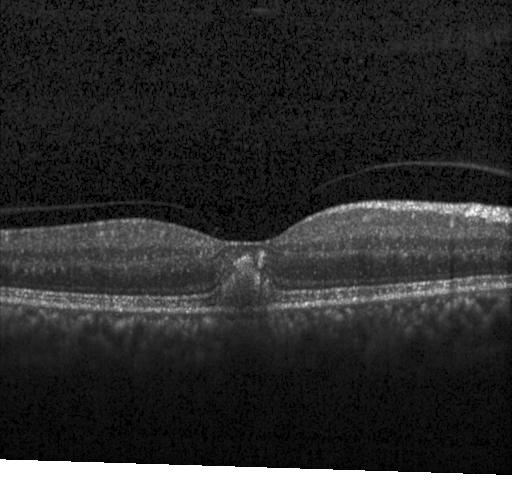
Macular OCT demonstrating choroidal neovascularization (CNV).